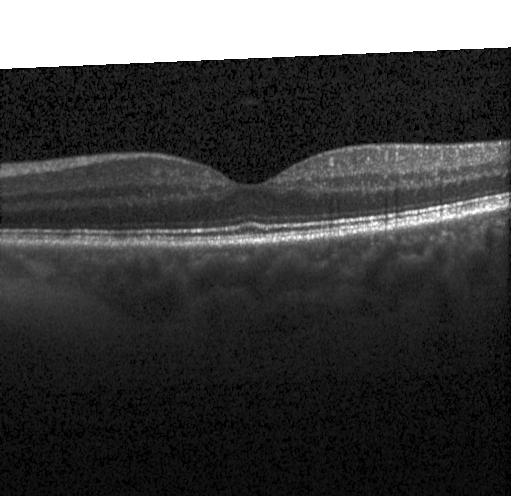

Retinal OCT B-scan — Neither choroidal neovascularization, diabetic macular edema, nor drusen.